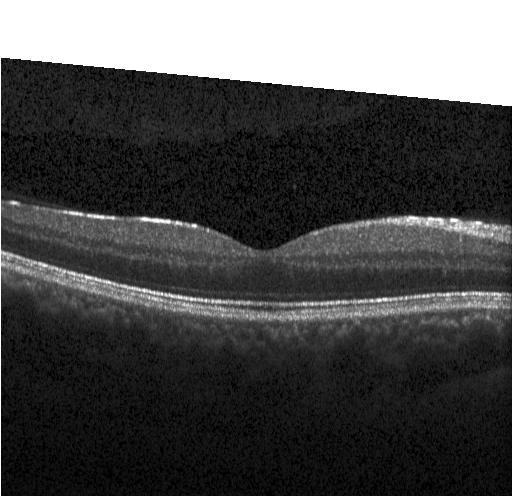

Retinal OCT cross-section showing no choroidal neovascularization, diabetic macular edema, or drusen.